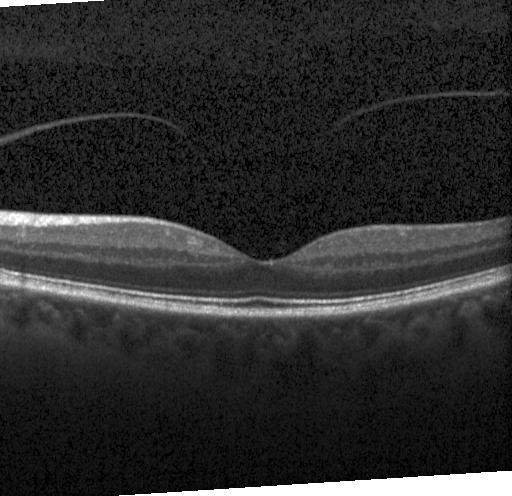 Dx: no choroidal neovascularization, no diabetic macular edema, and no drusen.